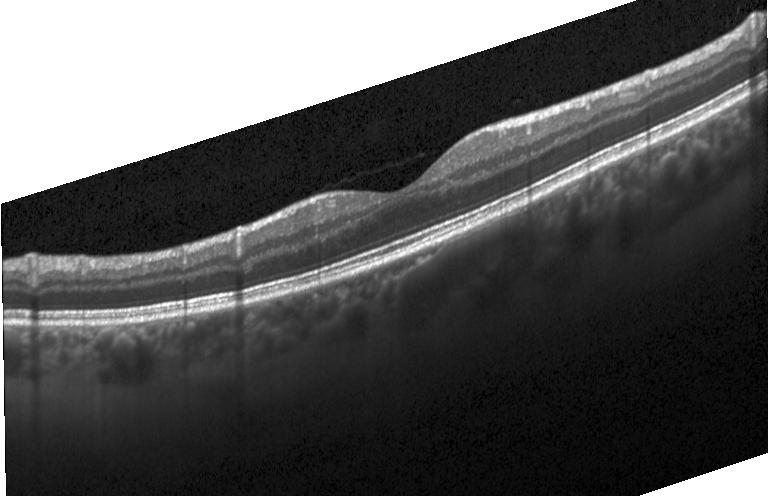

Fovea-centered; spectral-domain OCT; Heidelberg Spectralis OCT system; OCT line scan — Macular OCT: no choroidal neovascularization, diabetic macular edema, or drusen.